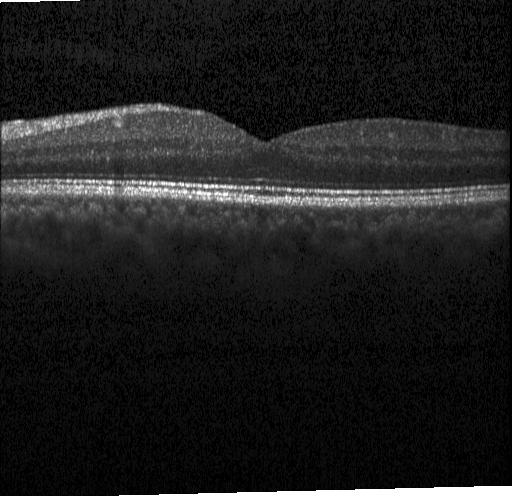

SD-OCT. Retinal OCT cross-section. Acquired on a Heidelberg Spectralis
No evidence of CNV, DME, or drusen.